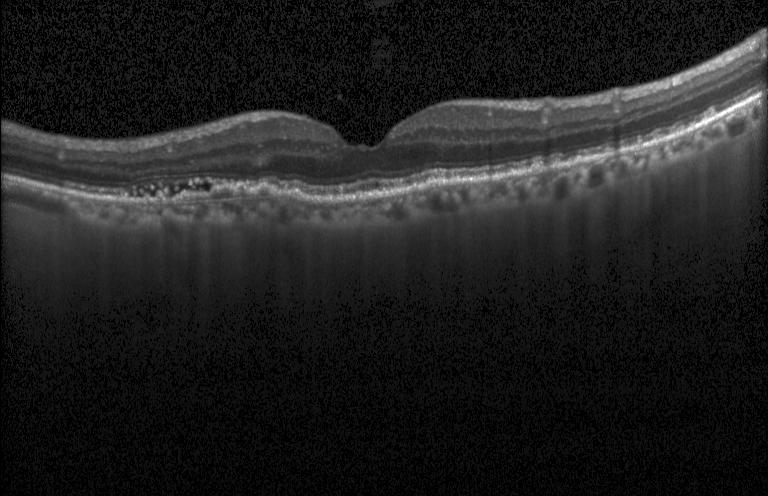

Retinal OCT cross-section showing a choroidal neovascular membrane.